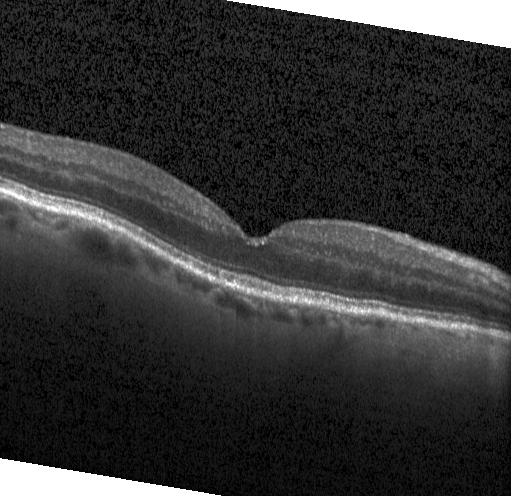
Macular OCT: no CNV, DME, or drusen.